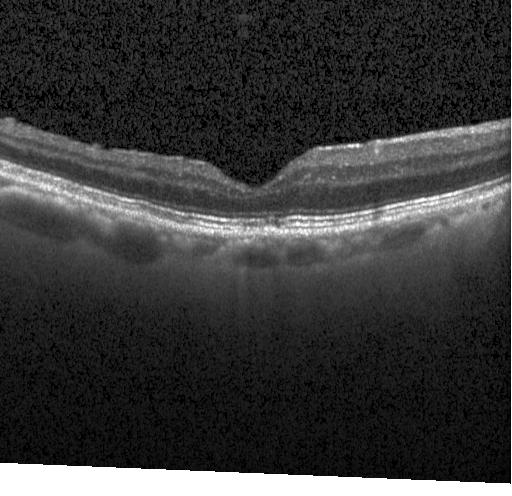
Retinal OCT B-scan.
Finding: no choroidal neovascularization, no diabetic macular edema, and no drusen.